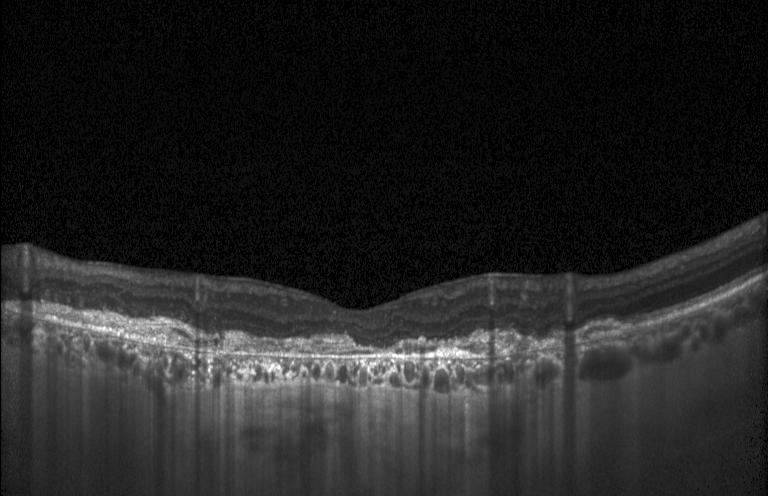
Finding: a choroidal neovascular membrane.